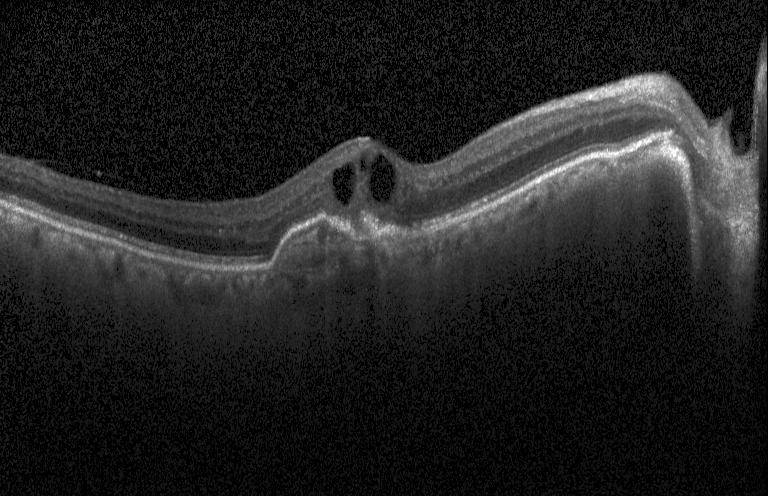

Heidelberg Spectralis OCT system · OCT line scan · horizontal scan through the fovea
Diagnosis: a choroidal neovascular membrane.